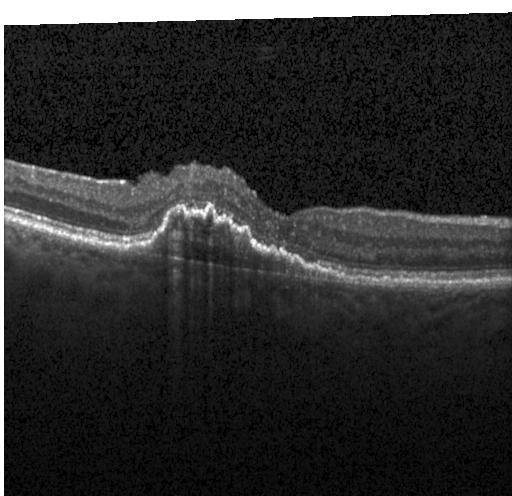

SD-OCT. Fovea-centered. Retinal OCT B-scan
A choroidal neovascular membrane.